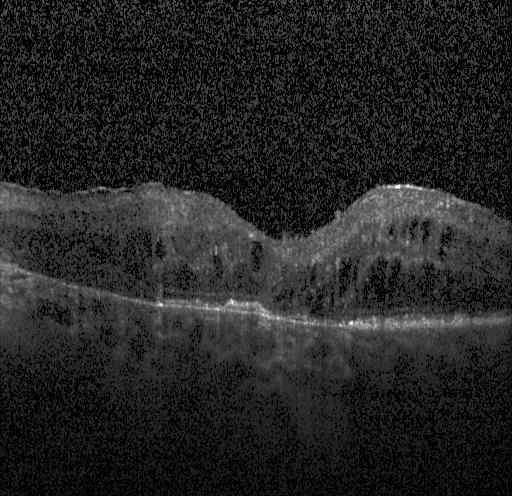 Retinal OCT cross-section. Diagnosis: choroidal neovascularization (CNV).